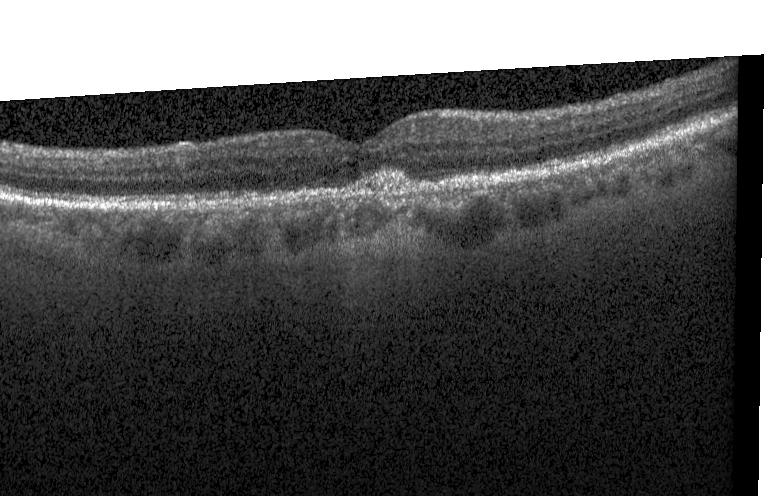

OCT line scan. Macular scan. SD-OCT. Heidelberg Spectralis OCT system.
Diagnosis: a choroidal neovascular membrane.